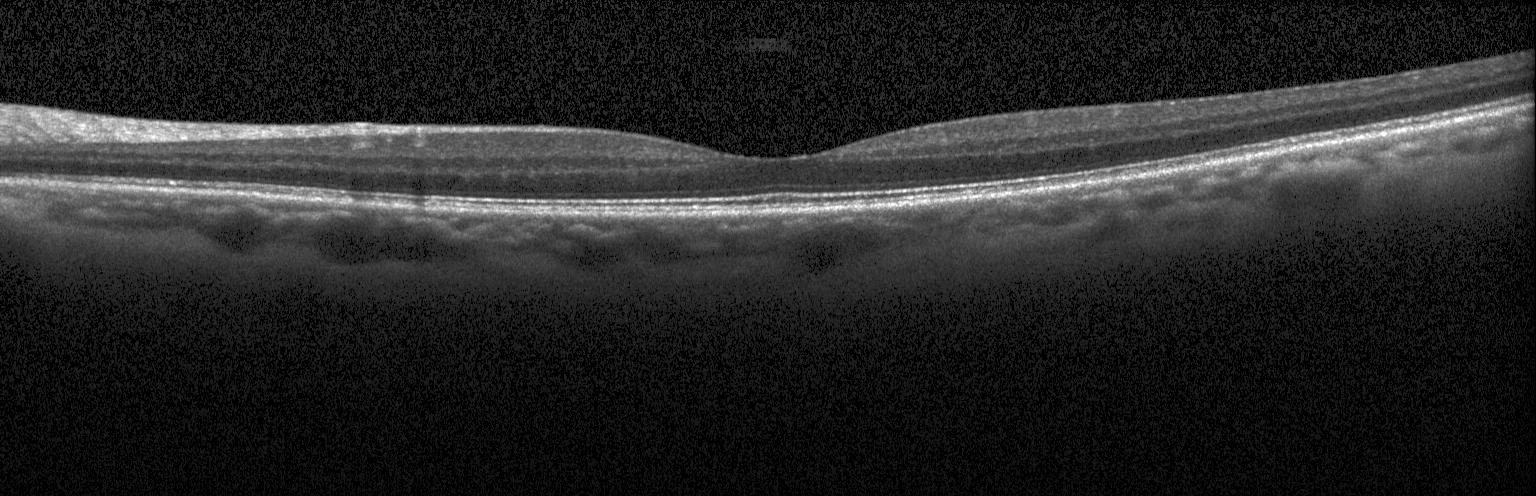

Optical coherence tomography scan, Heidelberg Spectralis, through the macula
This B-scan demonstrates no choroidal neovascularization, diabetic macular edema, or drusen.